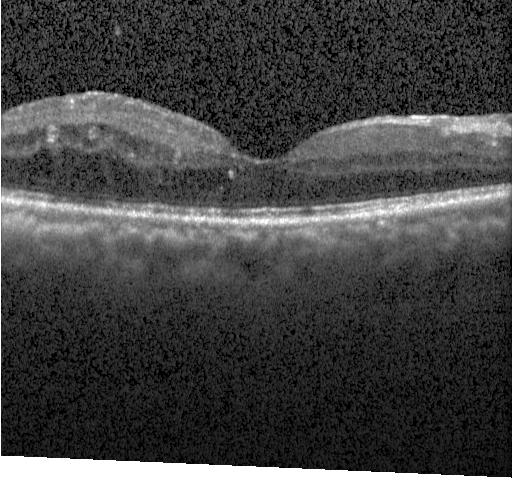
OCT B-scan · SD-OCT. The scan shows diabetic macular edema.